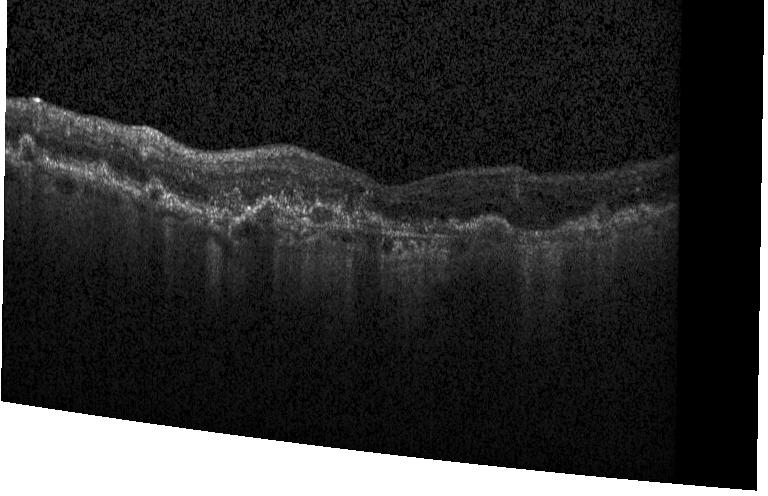
OCT B-scan showing a choroidal neovascular membrane.